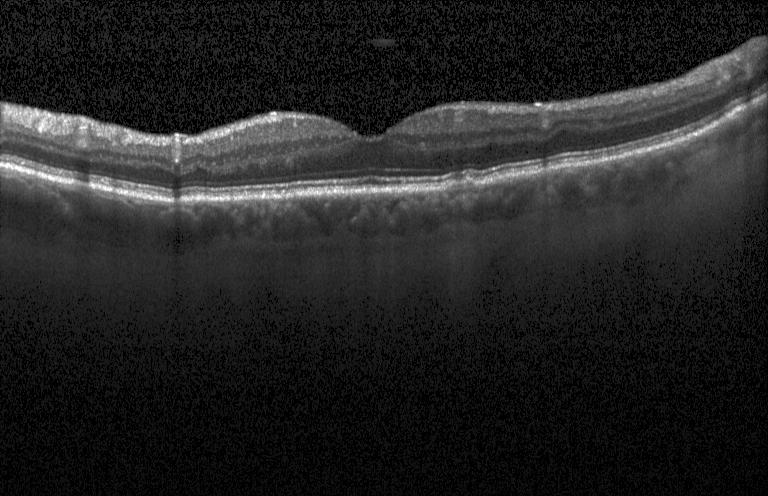
Optical coherence tomography scan. Spectral-domain optical coherence tomography. Heidelberg Spectralis. The scan shows multiple drusen.